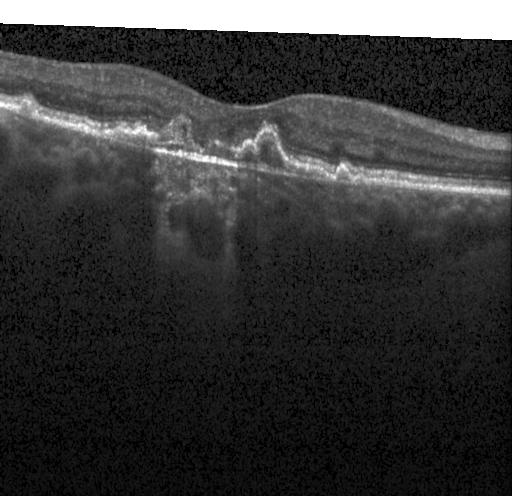

Impression: a choroidal neovascular membrane.